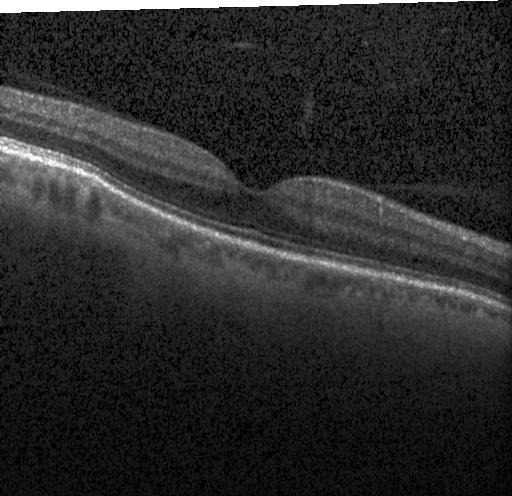

Macular scan. OCT B-scan. No choroidal neovascularization, diabetic macular edema, or drusen.